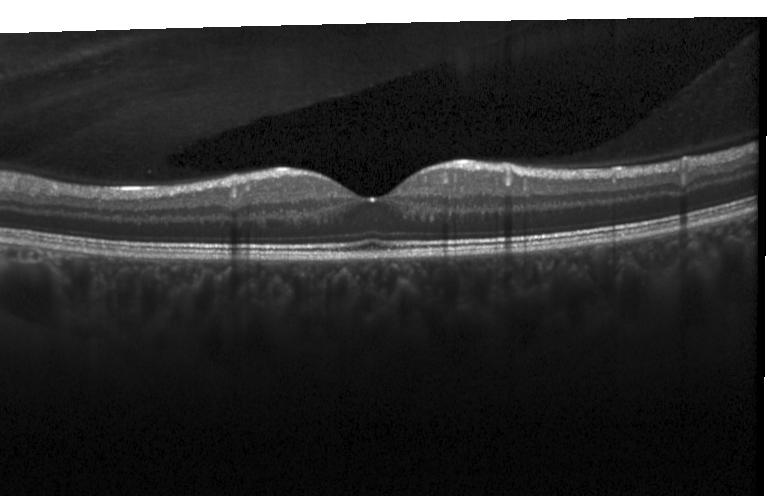

No evidence of choroidal neovascularization, diabetic macular edema, or drusen.